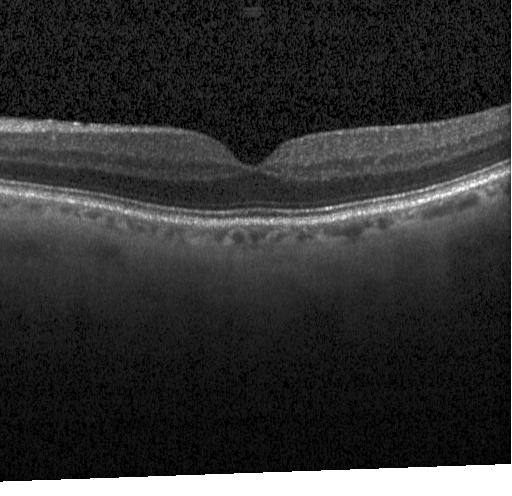
OCT line scan — Assessment: neither choroidal neovascularization, diabetic macular edema, nor drusen.